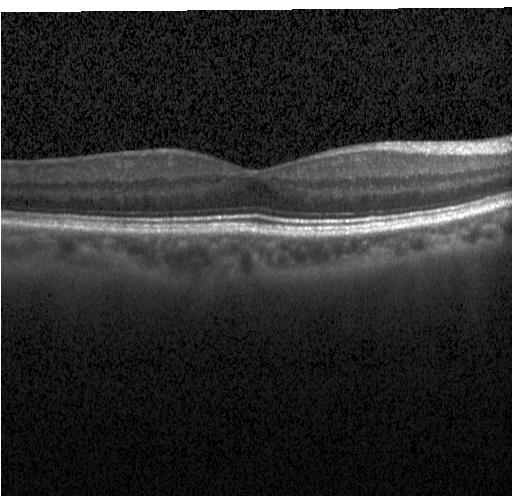

Macular OCT: no choroidal neovascularization, no diabetic macular edema, and no drusen.